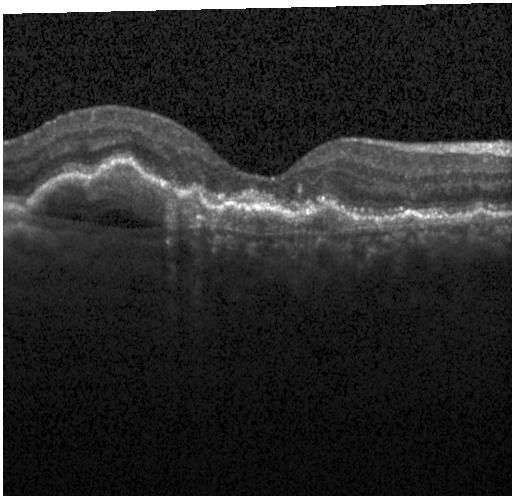 Optical coherence tomography B-scan. CNV.